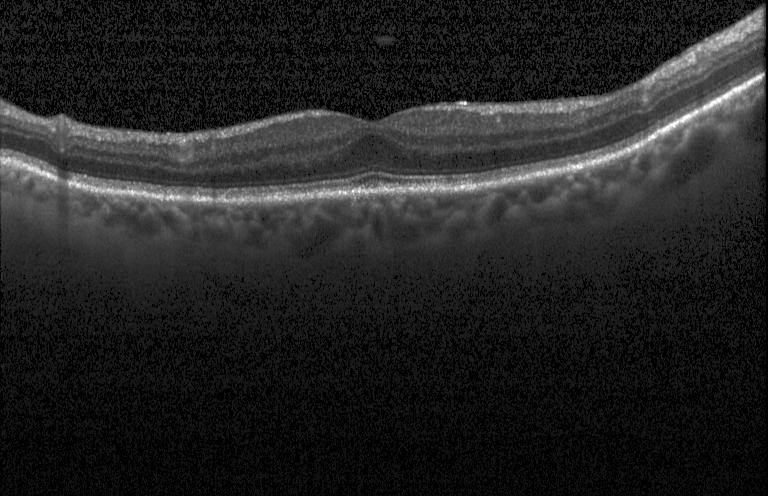

Dx: neither choroidal neovascularization, diabetic macular edema, nor drusen.